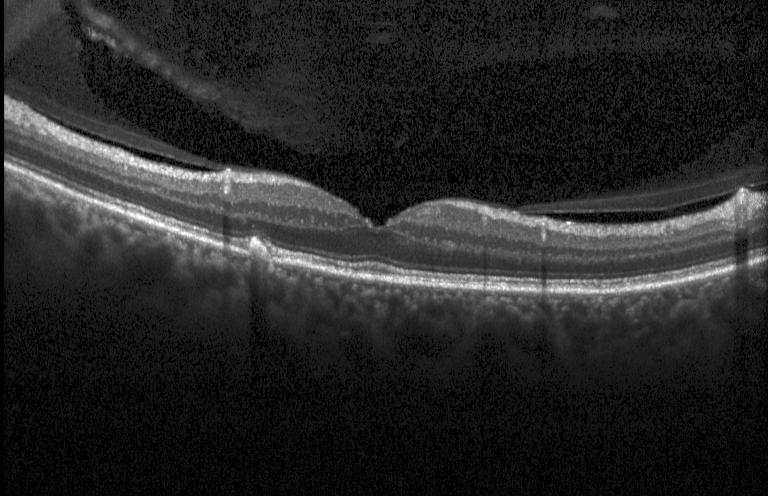

OCT scan showing drusen.